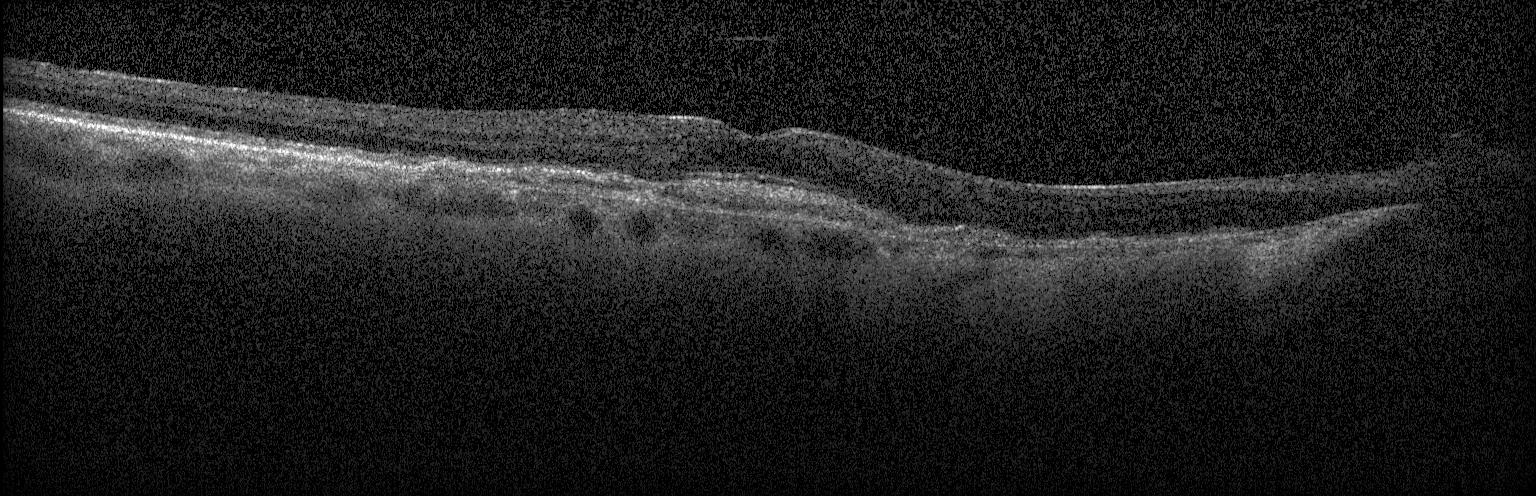 Optical coherence tomography B-scan; Heidelberg Spectralis OCT system — Dx: a choroidal neovascular membrane.